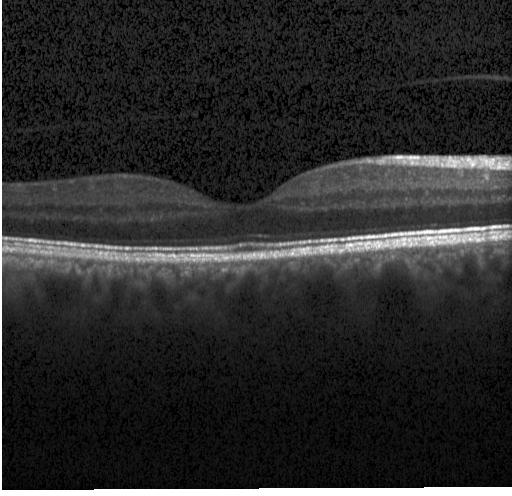 Retinal OCT B-scan. Fovea-centered
Diagnosis: no choroidal neovascularization, diabetic macular edema, or drusen.